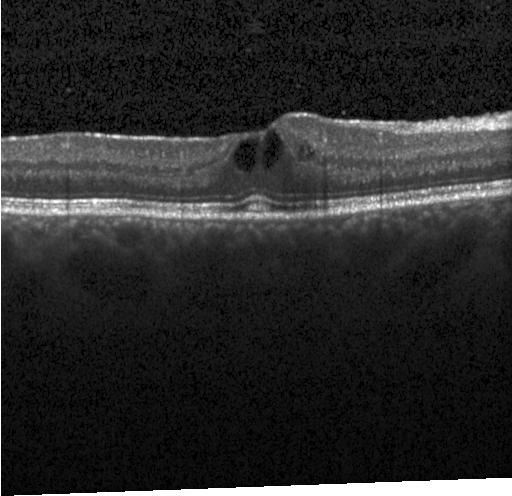

Optical coherence tomography B-scan. Diagnosis: DME.